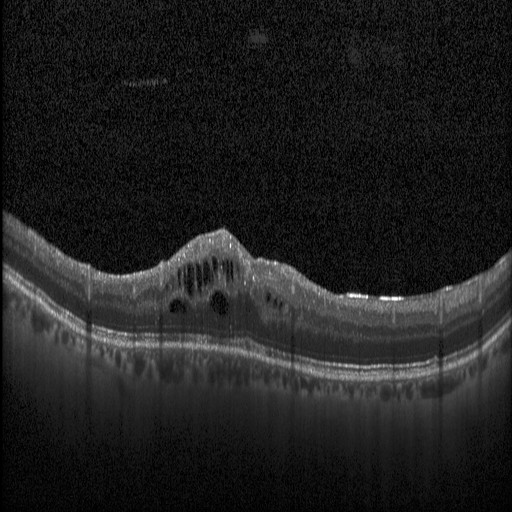

Retinal OCT B-scan; spectral-domain optical coherence tomography; centered on the fovea; Heidelberg Spectralis OCT system.
This B-scan demonstrates diabetic macular edema.